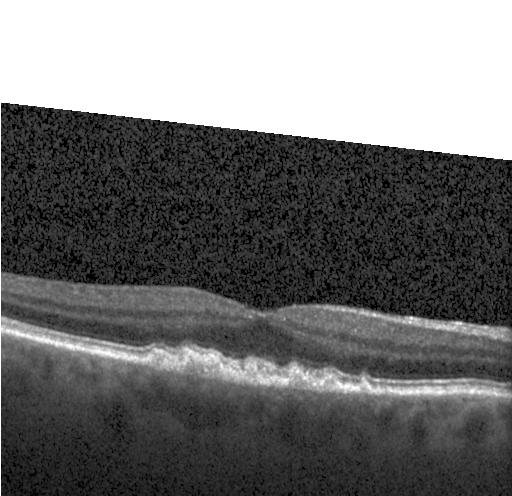
Finding: sub-RPE drusenoid deposits.